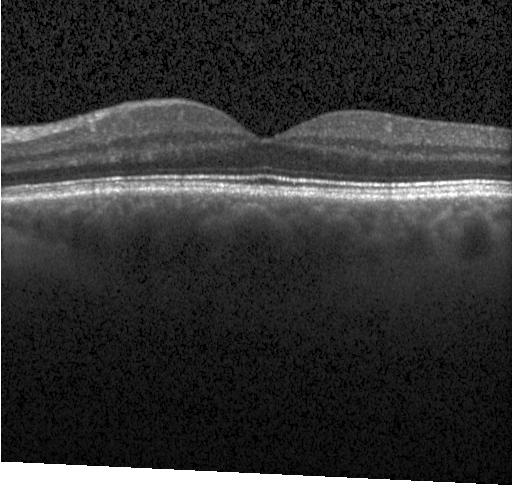 Spectral-domain optical coherence tomography · Heidelberg Spectralis OCT system · retinal OCT cross-section · through the macula
Macular OCT: no choroidal neovascularization, diabetic macular edema, or drusen.